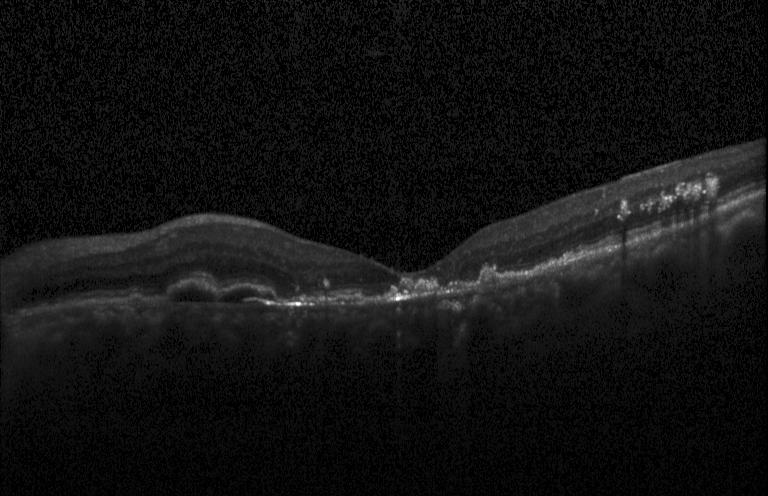 OCT B-scan. Through the macula. A choroidal neovascular membrane.